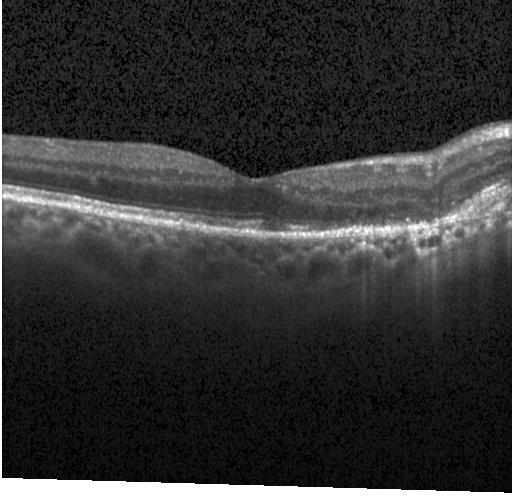
Optical coherence tomography scan. Acquired on a Heidelberg Spectralis.
Dx: a choroidal neovascular membrane.